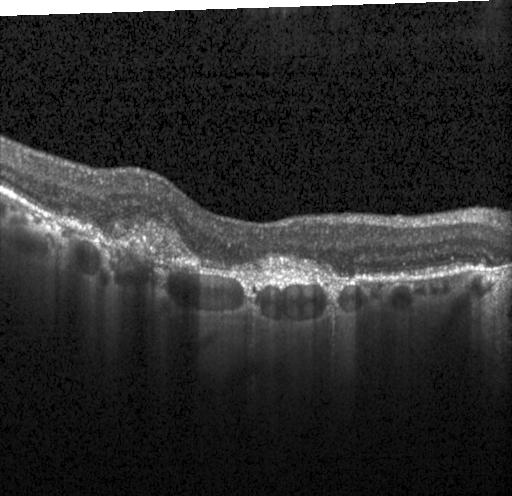

Optical coherence tomography scan.
This B-scan demonstrates a choroidal neovascular membrane.